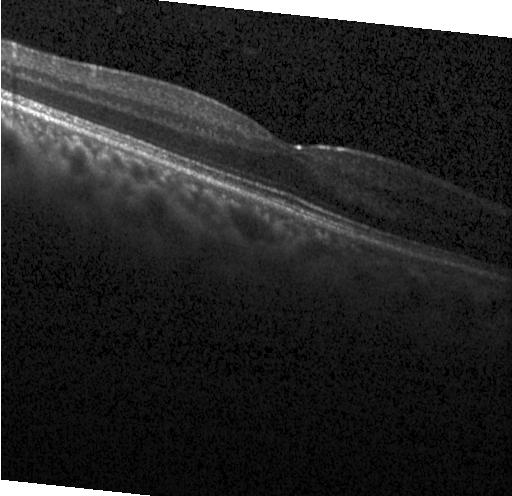 Retinal OCT cross-section; spectral-domain optical coherence tomography — Assessment: no evidence of choroidal neovascularization, diabetic macular edema, or drusen.